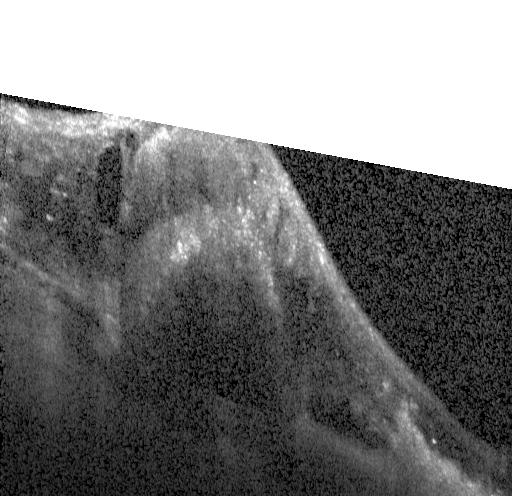 Fovea-centered, retinal OCT cross-section, Heidelberg Spectralis, spectral-domain OCT
Impression: choroidal neovascularization (CNV).